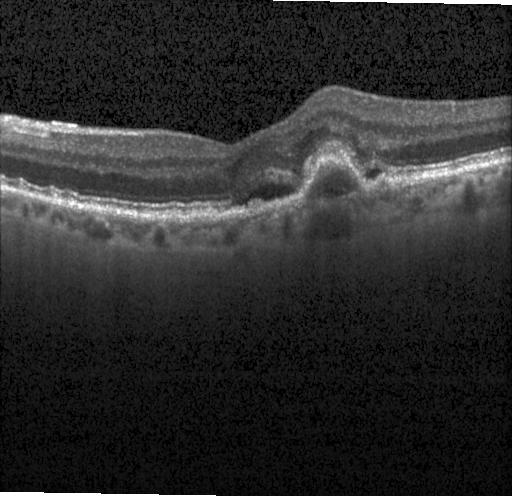
Retinal OCT cross-section — Macular OCT: a choroidal neovascular membrane.